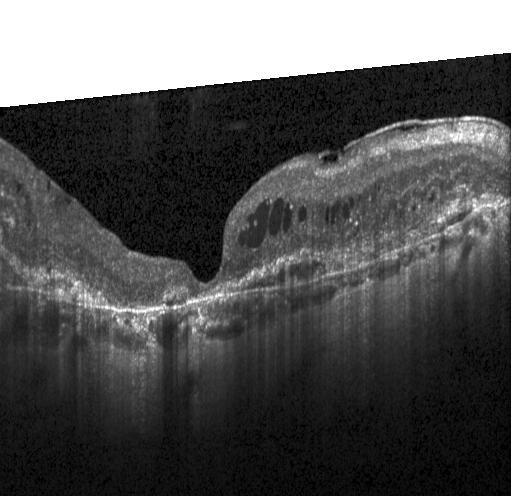

Centered on the fovea, SD-OCT, OCT line scan
Impression: a choroidal neovascular membrane.